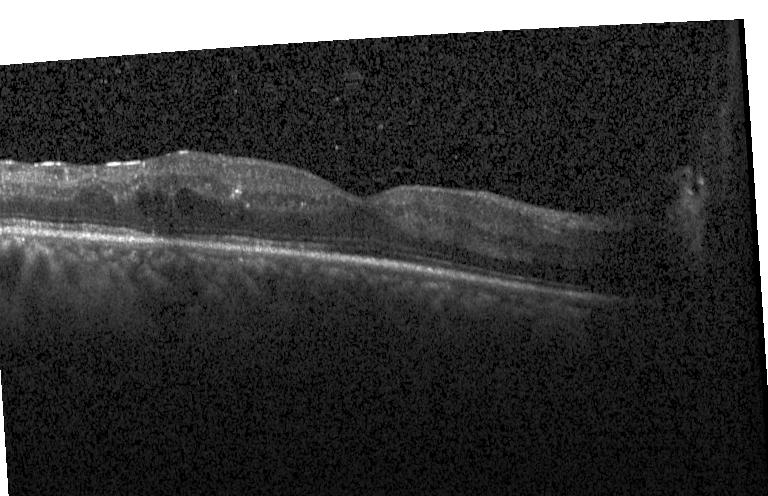 Retinal OCT B-scan · fovea-centered · acquired on a Heidelberg Spectralis
Impression: DME.